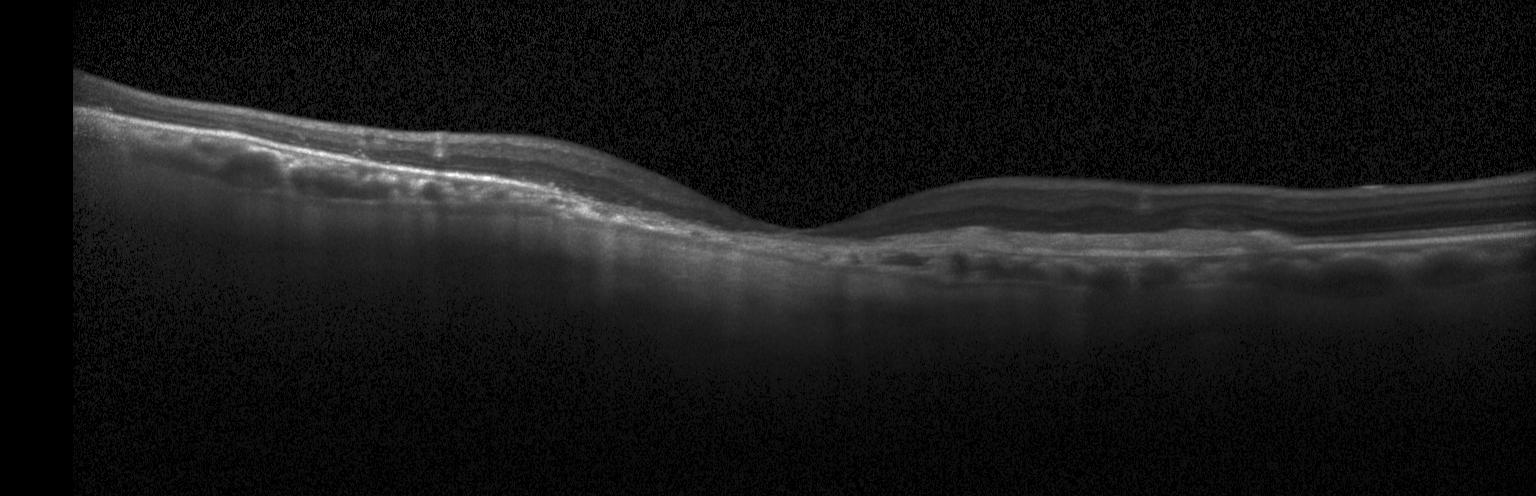

Fovea-centered, retinal OCT B-scan. Impression: choroidal neovascularization (CNV).